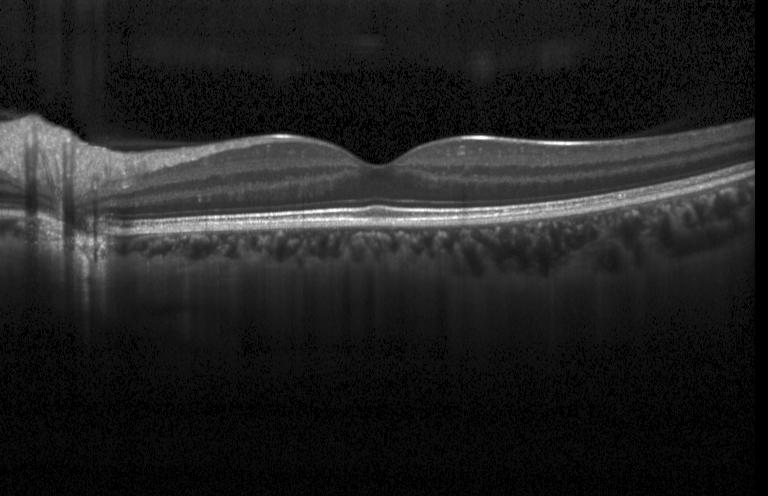

Dx: no choroidal neovascularization, no diabetic macular edema, and no drusen.